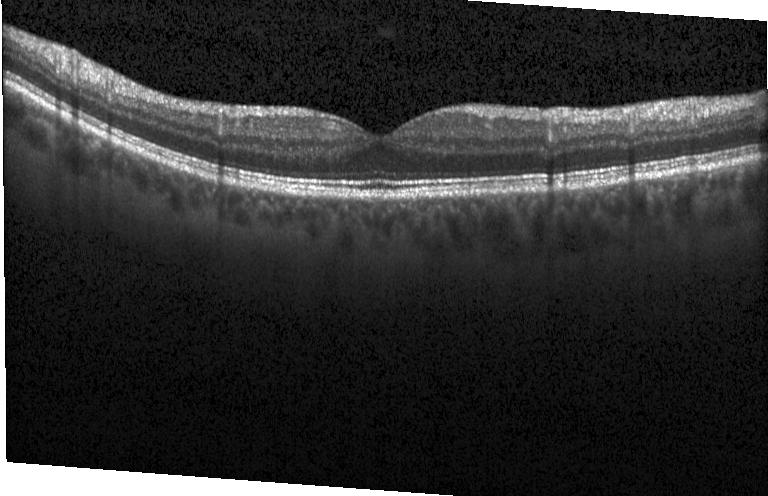 Horizontal scan through the fovea, OCT B-scan.
This B-scan demonstrates no evidence of CNV, DME, or drusen.